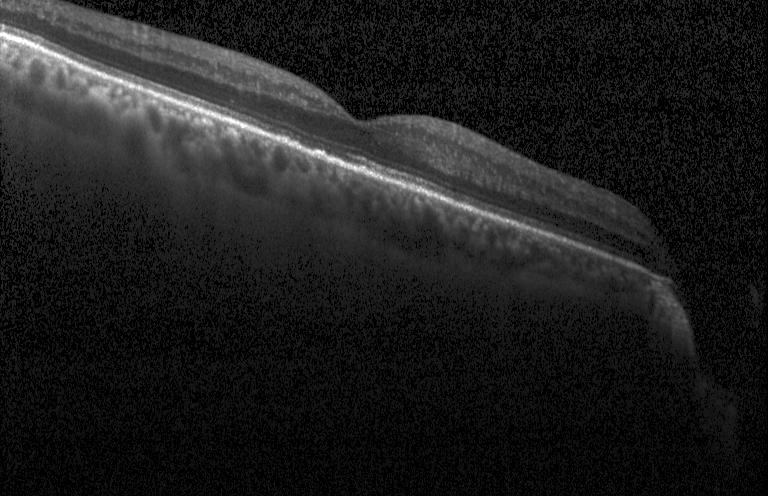

Macular OCT: neither CNV, DME, nor drusen.